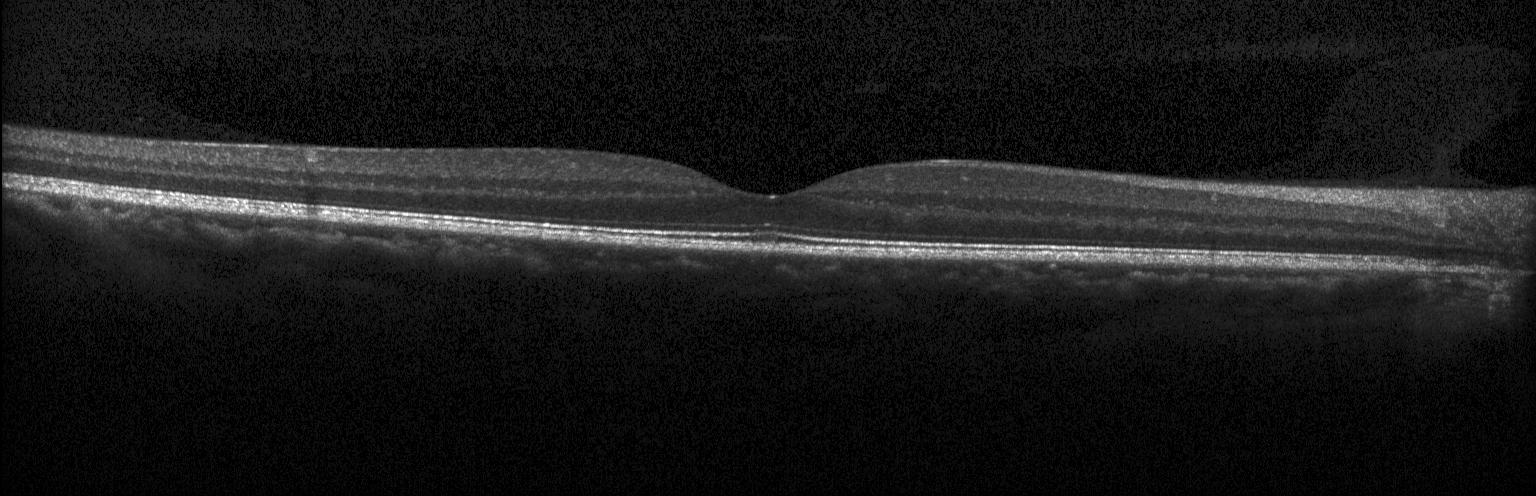

Fovea-centered; spectral-domain OCT; Heidelberg Spectralis; optical coherence tomography scan. OCT finding: no choroidal neovascularization, diabetic macular edema, or drusen.